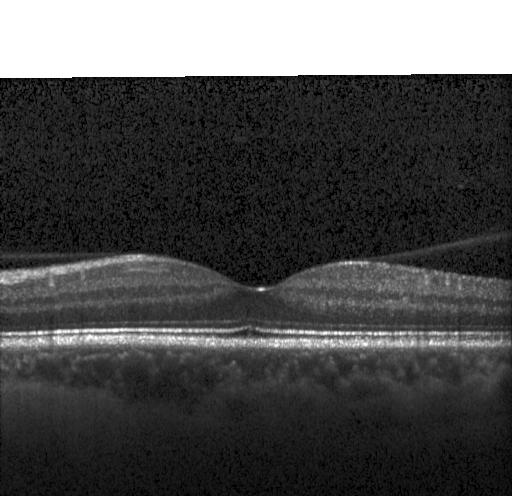 Impression: neither CNV, DME, nor drusen.